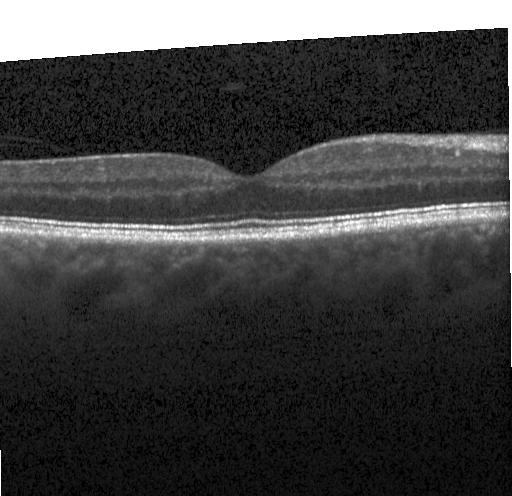

Diagnosis: no evidence of choroidal neovascularization, diabetic macular edema, or drusen.